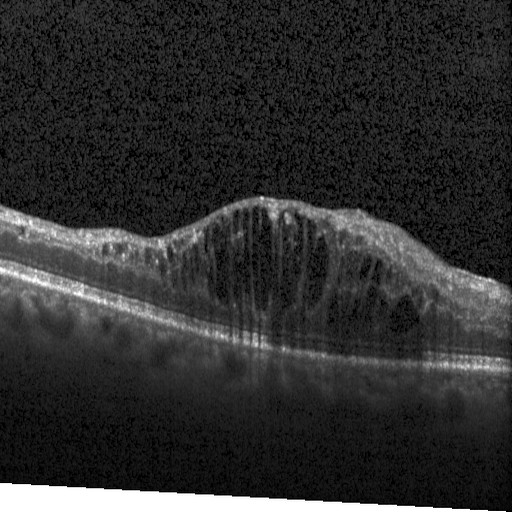
This B-scan demonstrates diabetic macular edema.